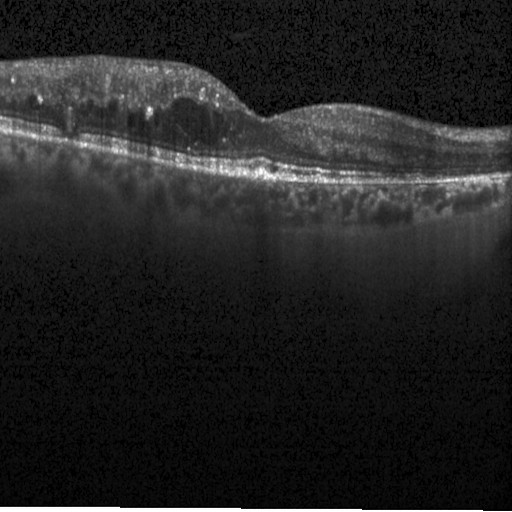 Optical coherence tomography B-scan, macular scan, SD-OCT. Diagnosis: diabetic macular edema (DME).